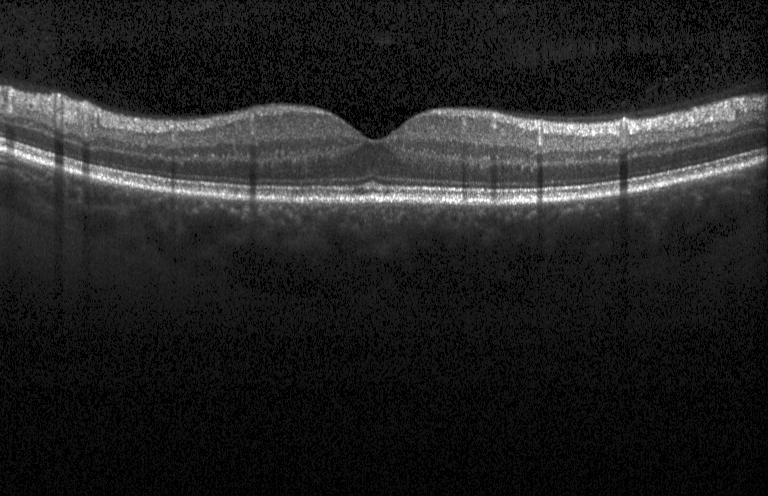

Dx: neither choroidal neovascularization, diabetic macular edema, nor drusen.